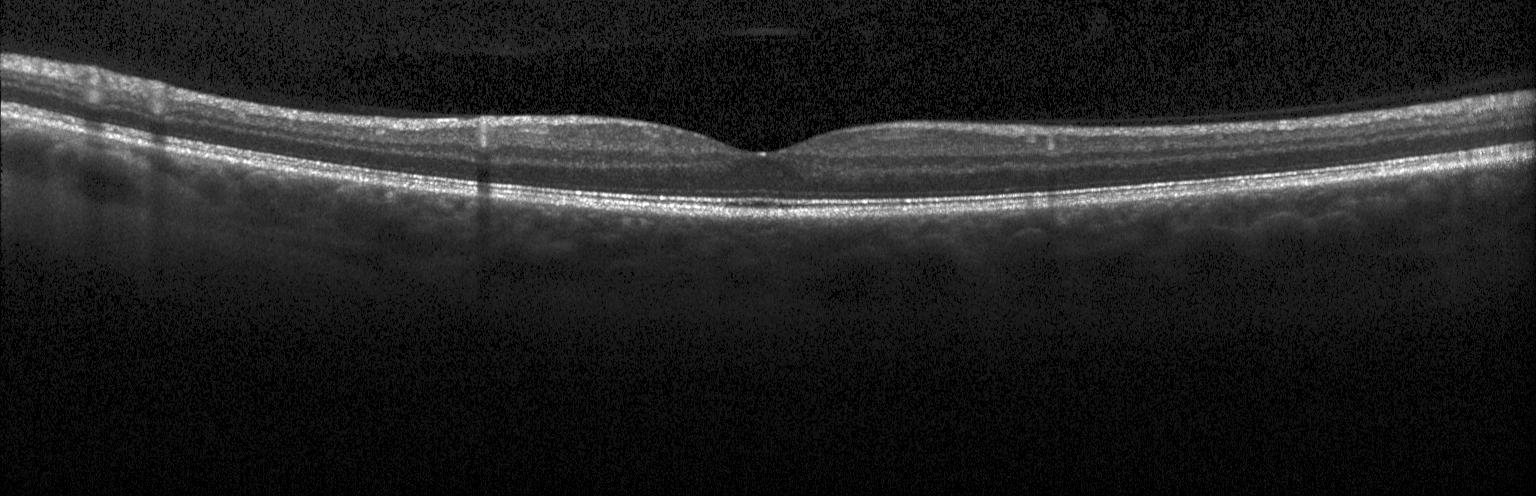
The scan shows no CNV, no DME, and no drusen.